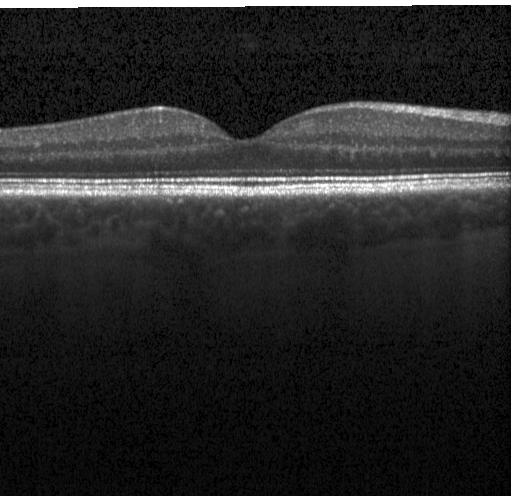 Dx: no evidence of choroidal neovascularization, diabetic macular edema, or drusen.